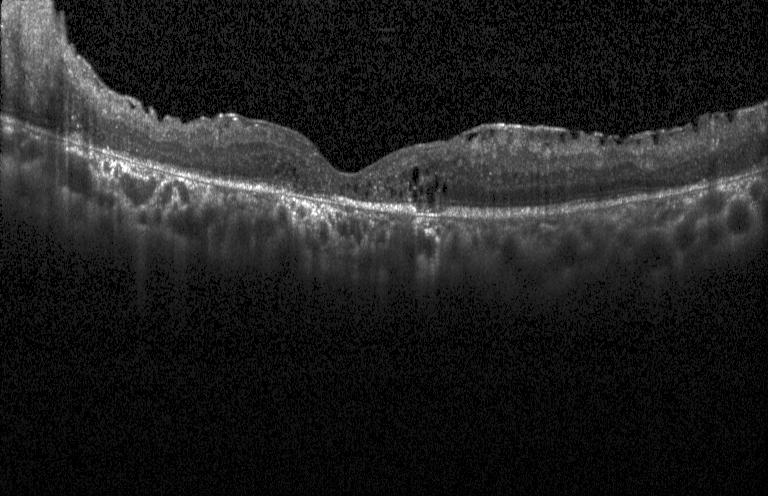
Macular OCT demonstrating CNV.